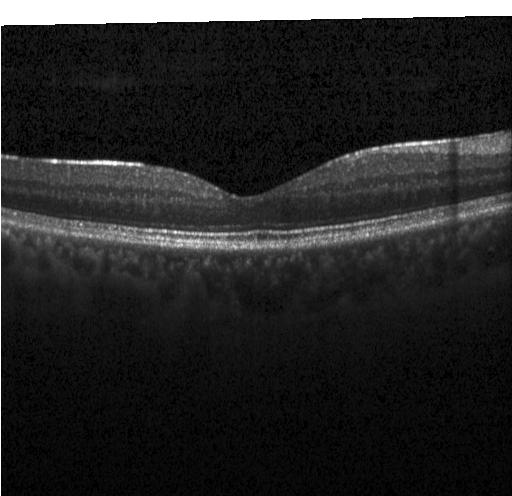
Diagnosis: neither CNV, DME, nor drusen.